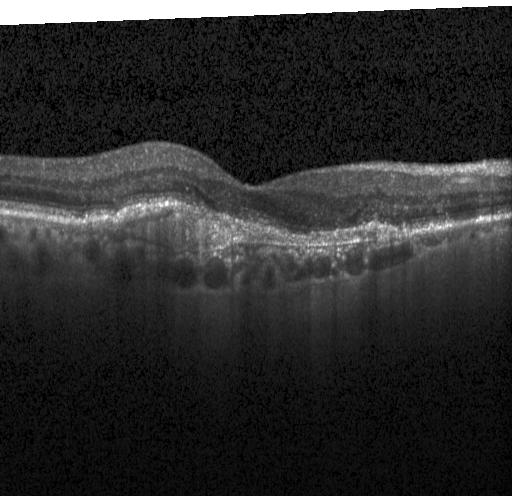

SD-OCT, centered on the fovea, optical coherence tomography B-scan, instrument: Heidelberg Spectralis — Assessment: choroidal neovascularization (CNV).